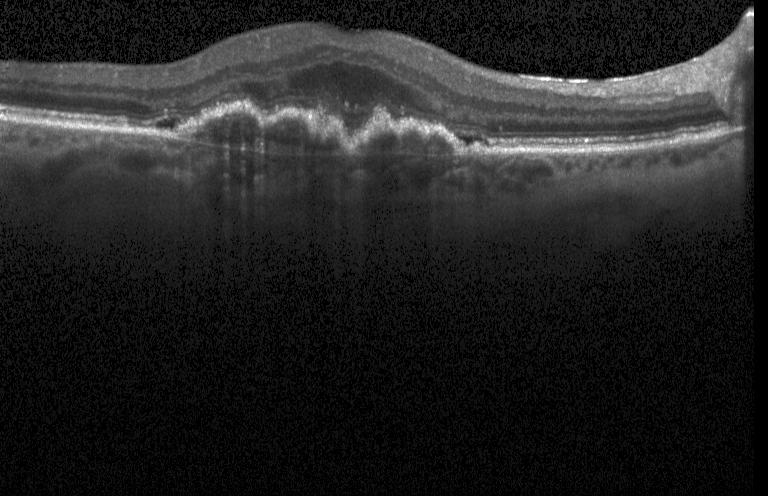 Dx: choroidal neovascularization.